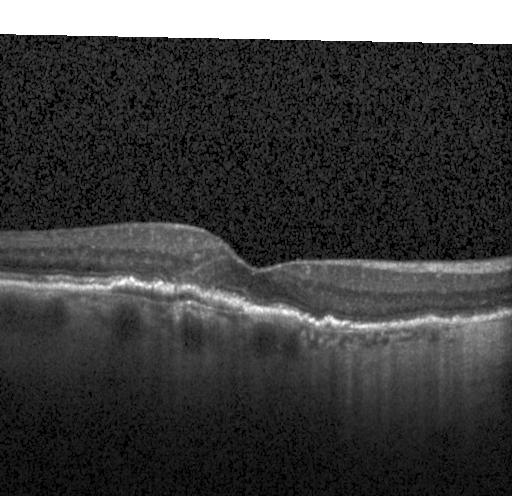

Optical coherence tomography scan. Assessment: a choroidal neovascular membrane.